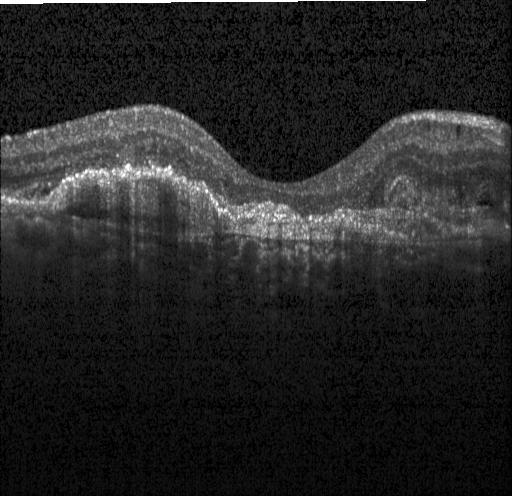 OCT B-scan; through the macula — Diagnosis: choroidal neovascularization.